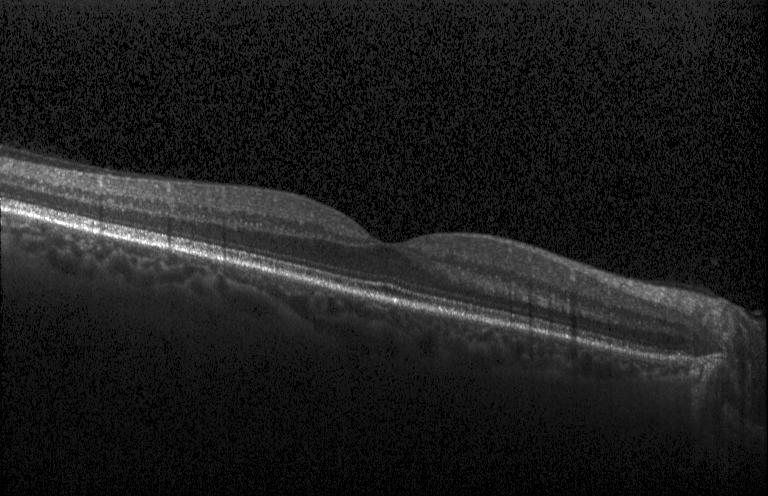

OCT finding: no evidence of choroidal neovascularization, diabetic macular edema, or drusen.